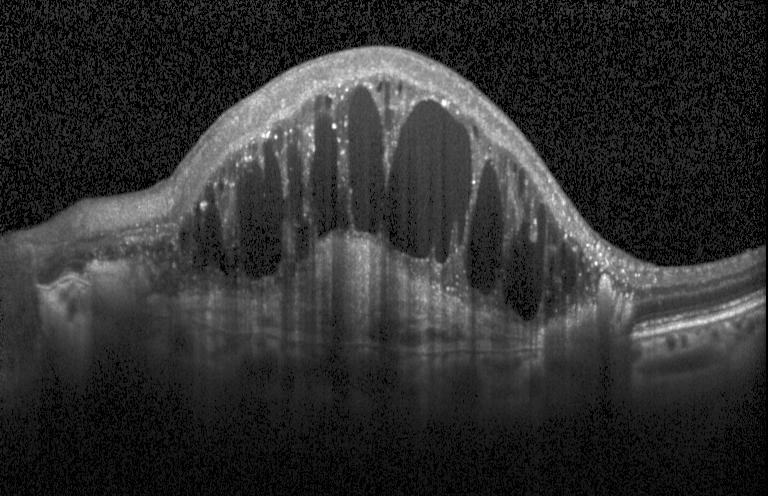

OCT finding: DME.